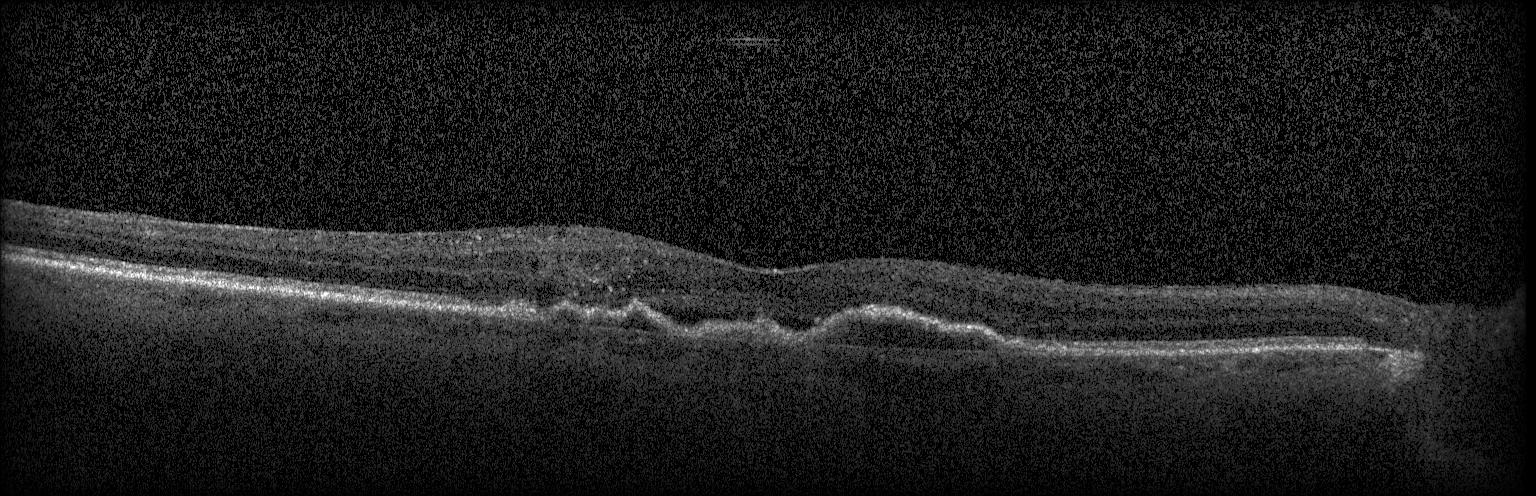
SD-OCT, retinal OCT cross-section, Heidelberg Spectralis, through the macula
Impression: a choroidal neovascular membrane.